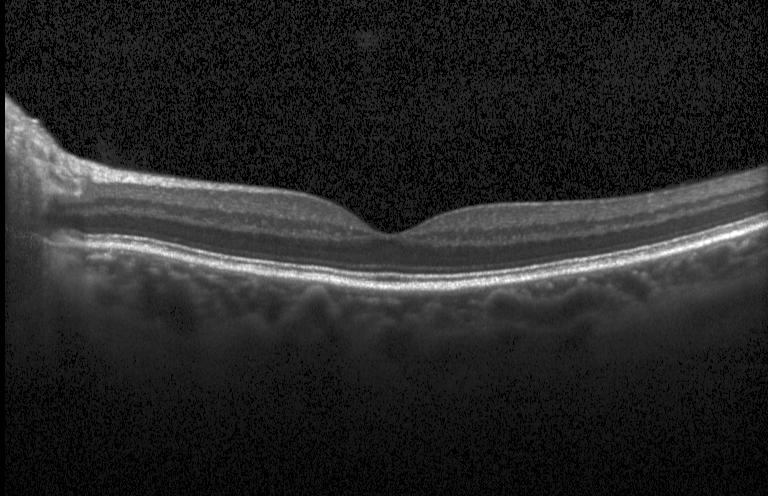
Retinal OCT B-scan; Heidelberg Spectralis; spectral-domain OCT; centered on the fovea. Finding: neither choroidal neovascularization, diabetic macular edema, nor drusen.